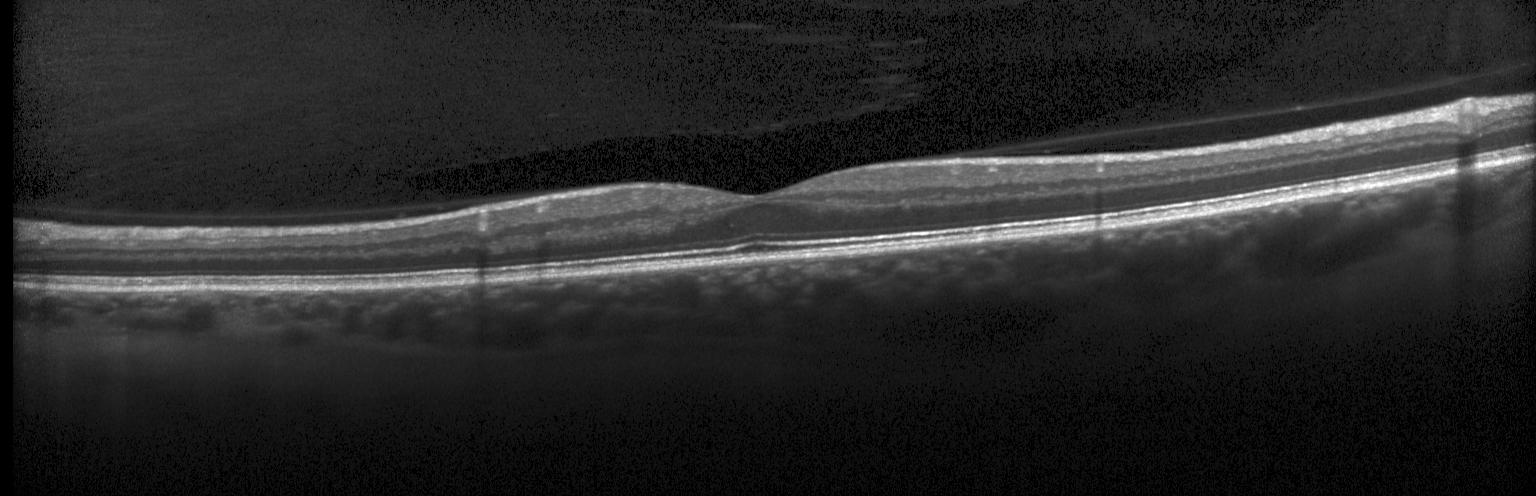 Finding: no CNV, no DME, and no drusen.